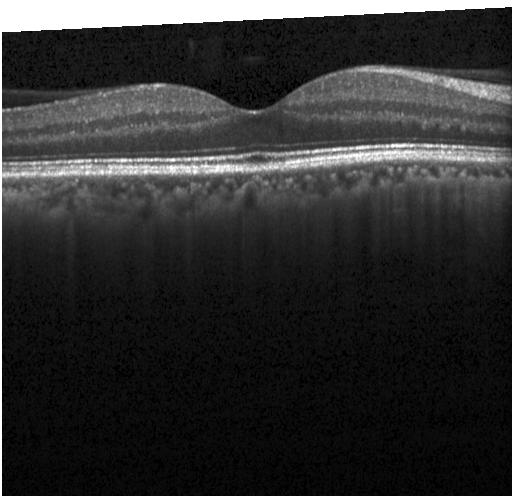 Optical coherence tomography B-scan. Finding: neither CNV, DME, nor drusen.